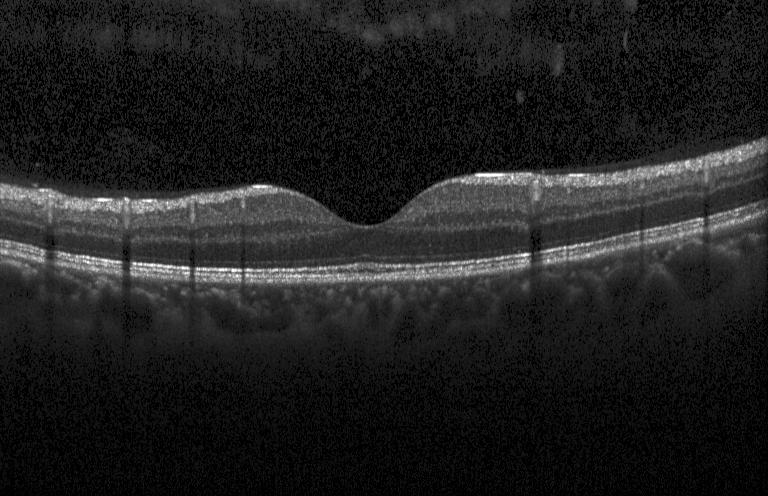
OCT B-scan, spectral-domain OCT.
Diagnosis: neither choroidal neovascularization, diabetic macular edema, nor drusen.